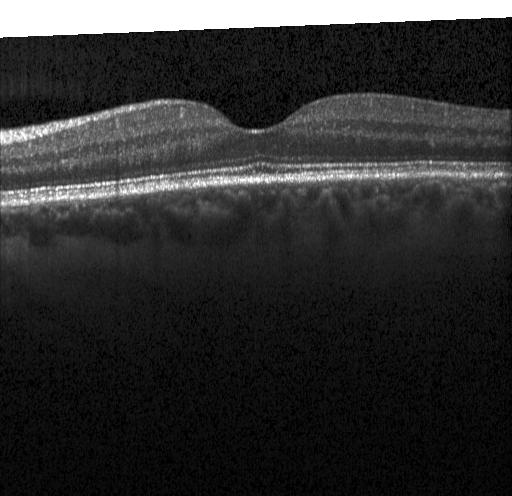 Retinal OCT B-scan — Diagnosis: neither CNV, DME, nor drusen.